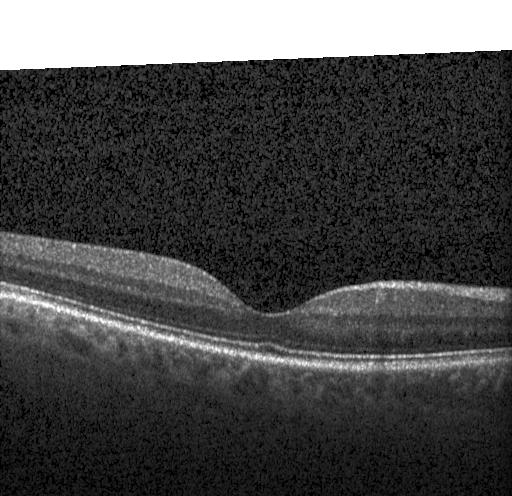
The scan shows no evidence of choroidal neovascularization, diabetic macular edema, or drusen.